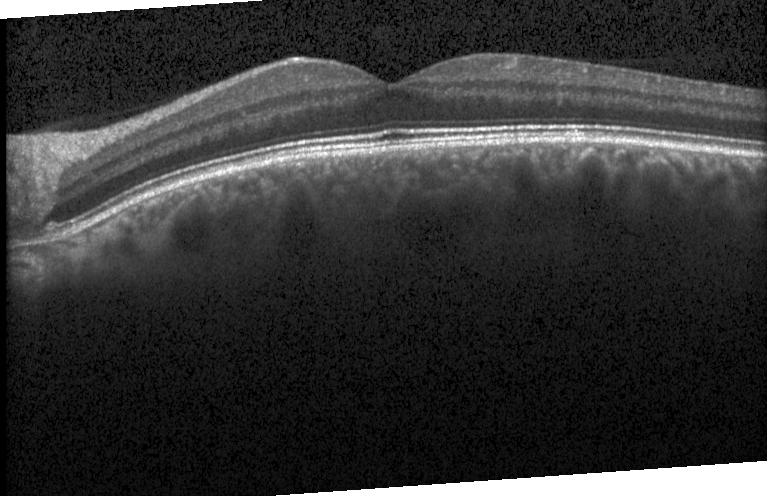 Dx: no choroidal neovascularization, no diabetic macular edema, and no drusen.